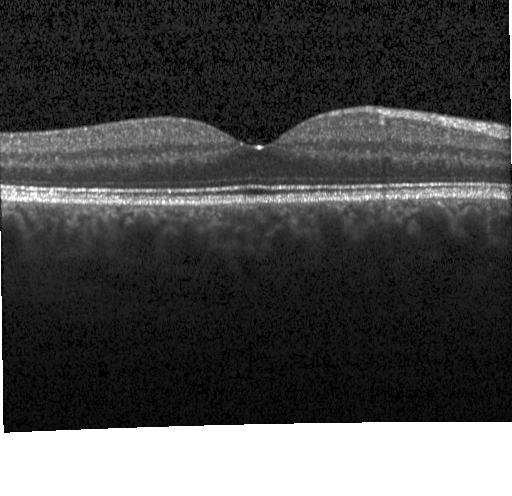

Acquired on a Heidelberg Spectralis; optical coherence tomography B-scan — Finding: no evidence of choroidal neovascularization, diabetic macular edema, or drusen.